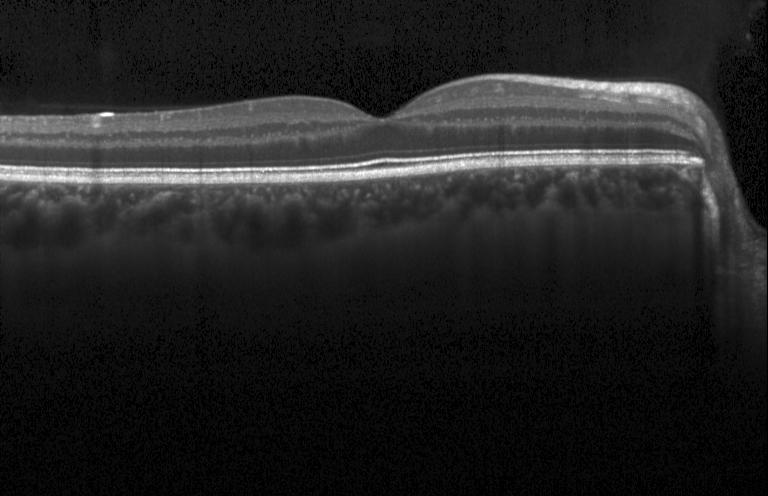

Macular scan; Heidelberg Spectralis; spectral-domain optical coherence tomography; optical coherence tomography scan — This B-scan demonstrates no choroidal neovascularization, diabetic macular edema, or drusen.